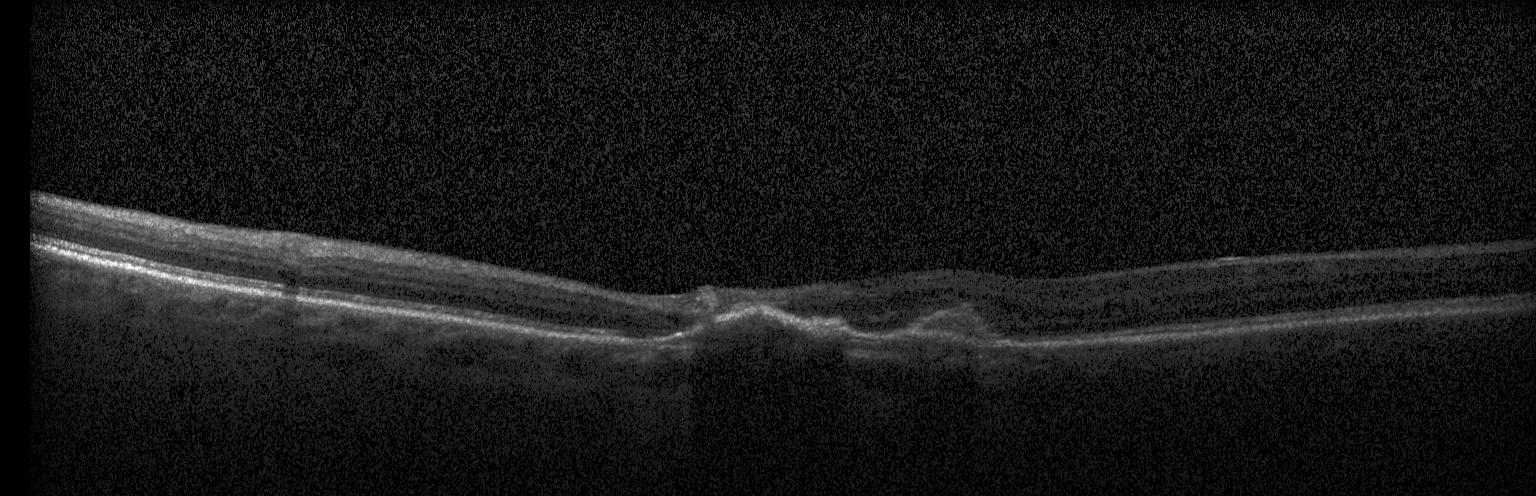

Optical coherence tomography B-scan — Diagnosis: a choroidal neovascular membrane.